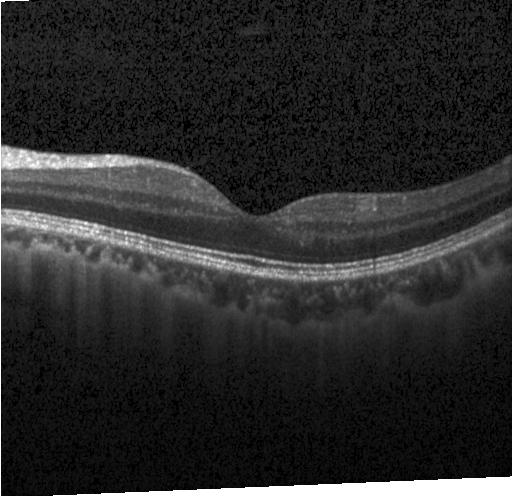 Macular OCT: no evidence of choroidal neovascularization, diabetic macular edema, or drusen.